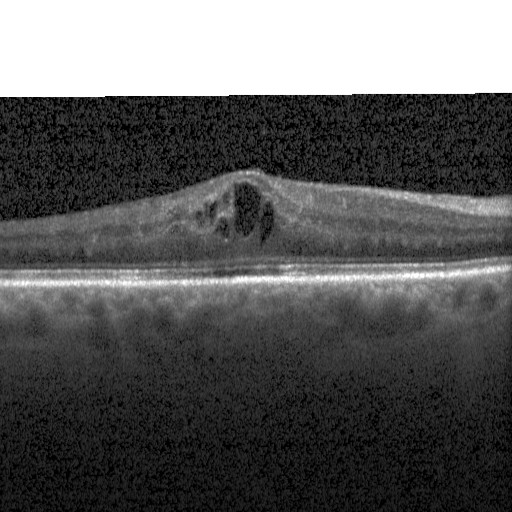 OCT finding: diabetic macular edema.